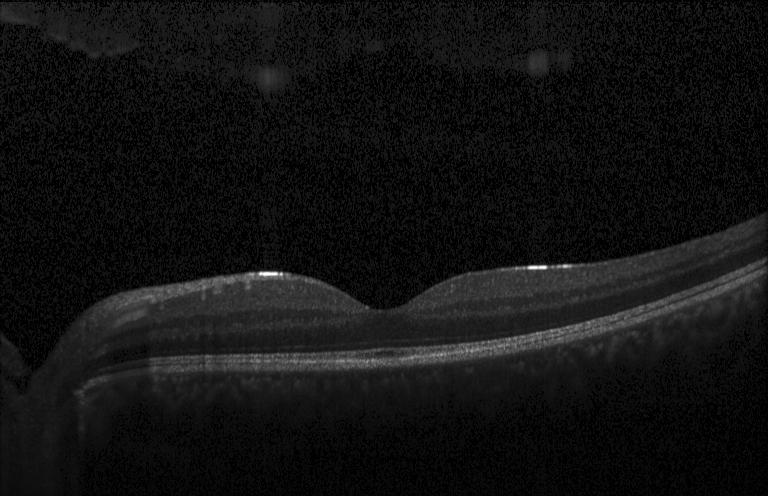
Retinal OCT cross-section.
Finding: no evidence of choroidal neovascularization, diabetic macular edema, or drusen.